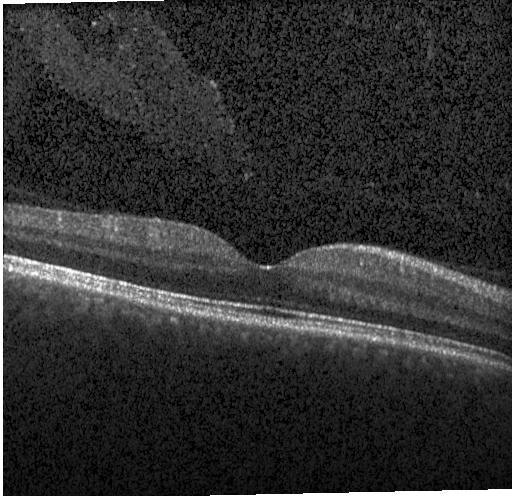 Macular OCT demonstrating neither CNV, DME, nor drusen.